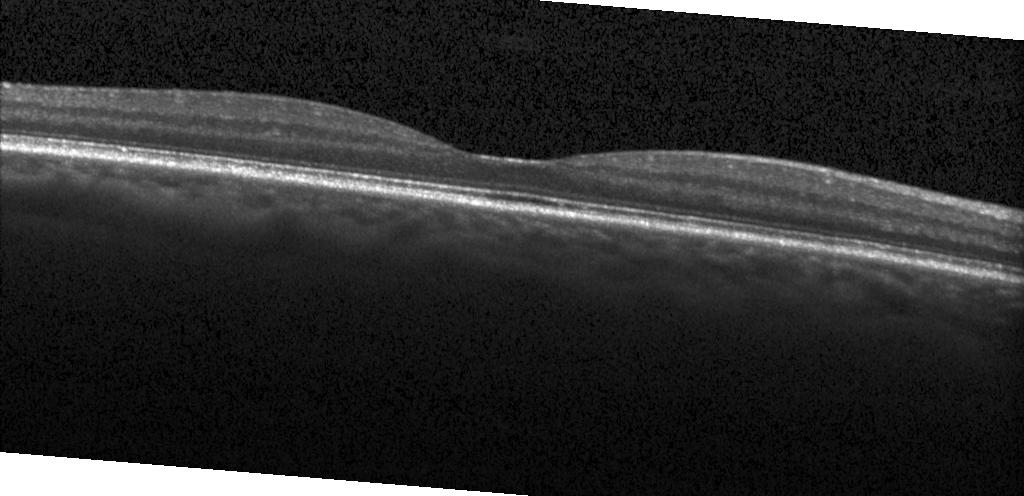 Spectral-domain OCT; horizontal scan through the fovea; optical coherence tomography B-scan
Assessment: no evidence of choroidal neovascularization, diabetic macular edema, or drusen.